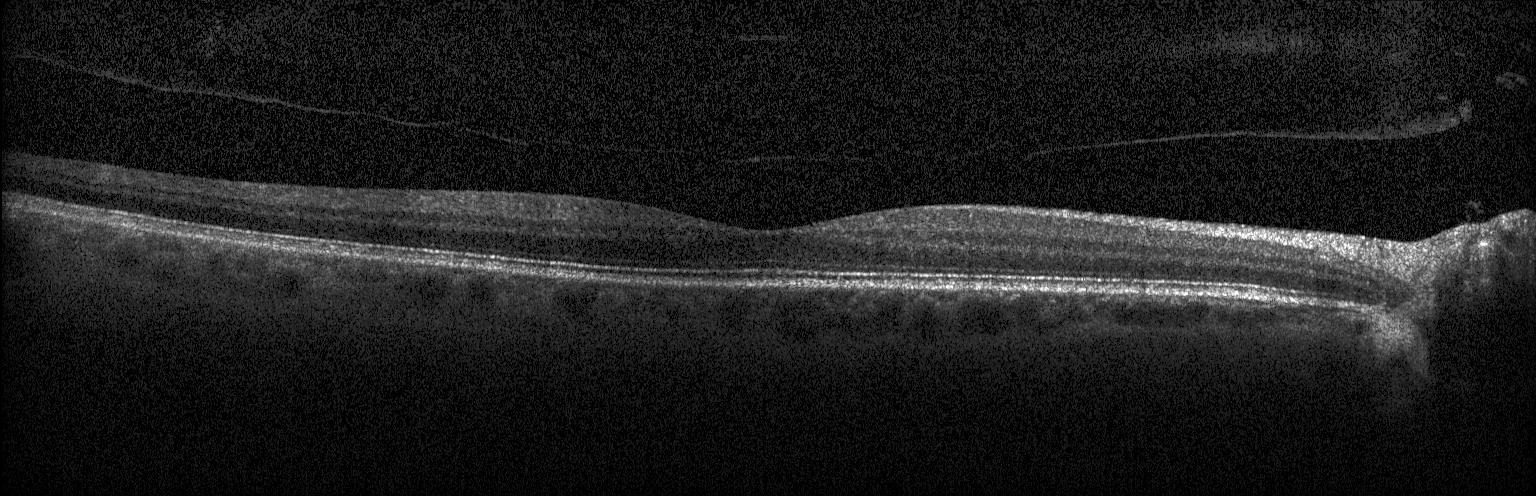

Optical coherence tomography scan.
Diagnosis: neither CNV, DME, nor drusen.